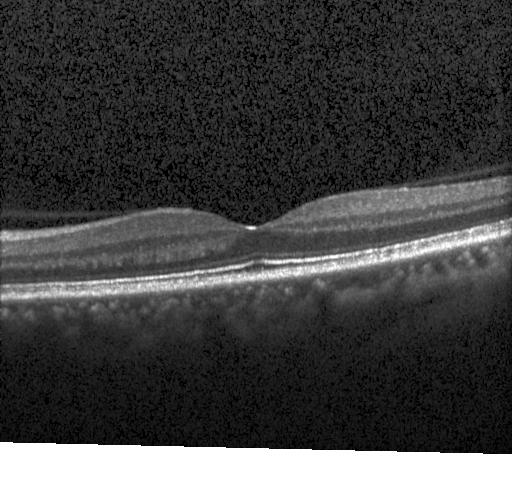 OCT line scan; Heidelberg Spectralis; macular scan; spectral-domain OCT — Impression: no CNV, DME, or drusen.